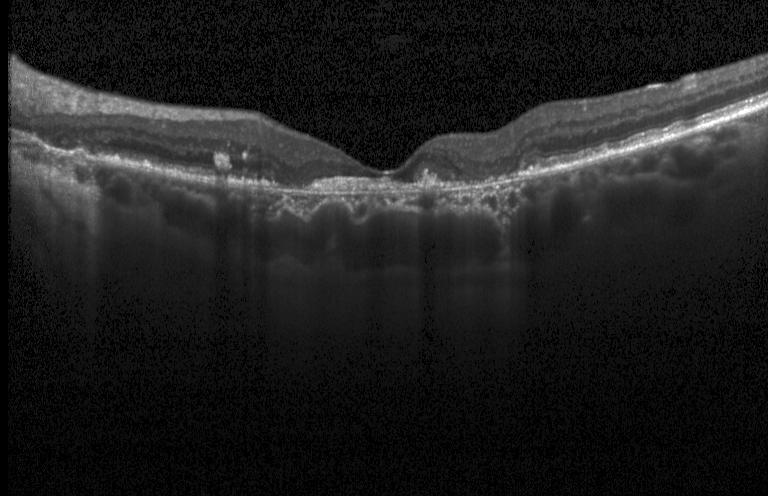
Macular OCT demonstrating a choroidal neovascular membrane.